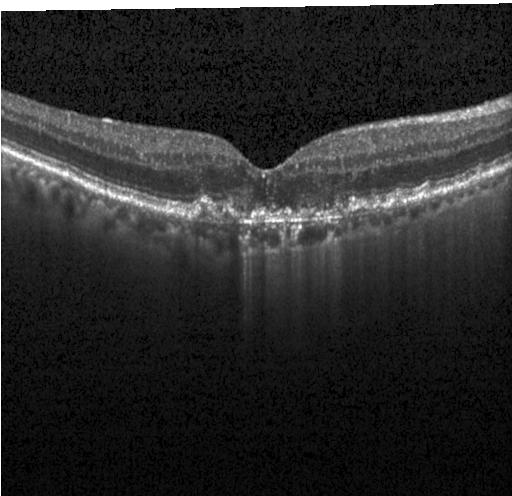 Heidelberg Spectralis OCT system; horizontal scan through the fovea; OCT B-scan. Diagnosis: a choroidal neovascular membrane.